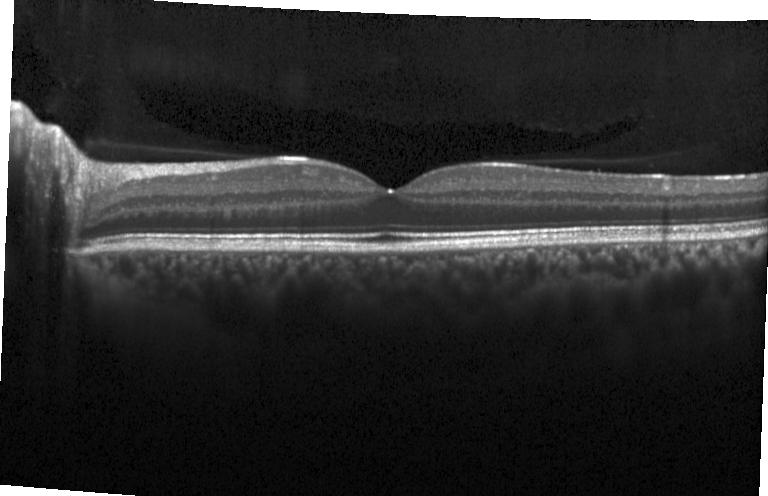 Horizontal scan through the fovea; OCT line scan — Dx: neither CNV, DME, nor drusen.